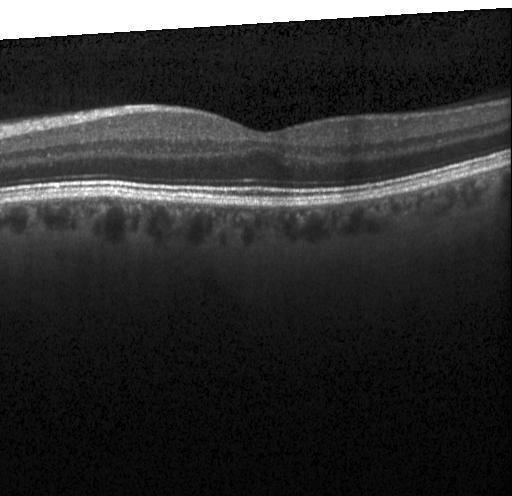

Impression: no CNV, no DME, and no drusen.